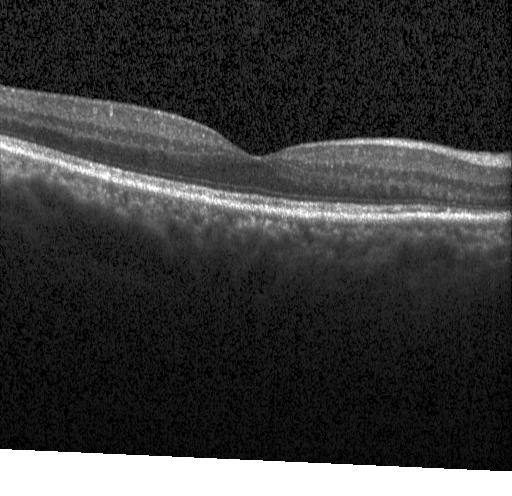 Horizontal scan through the fovea; instrument: Heidelberg Spectralis; optical coherence tomography scan. Finding: neither choroidal neovascularization, diabetic macular edema, nor drusen.